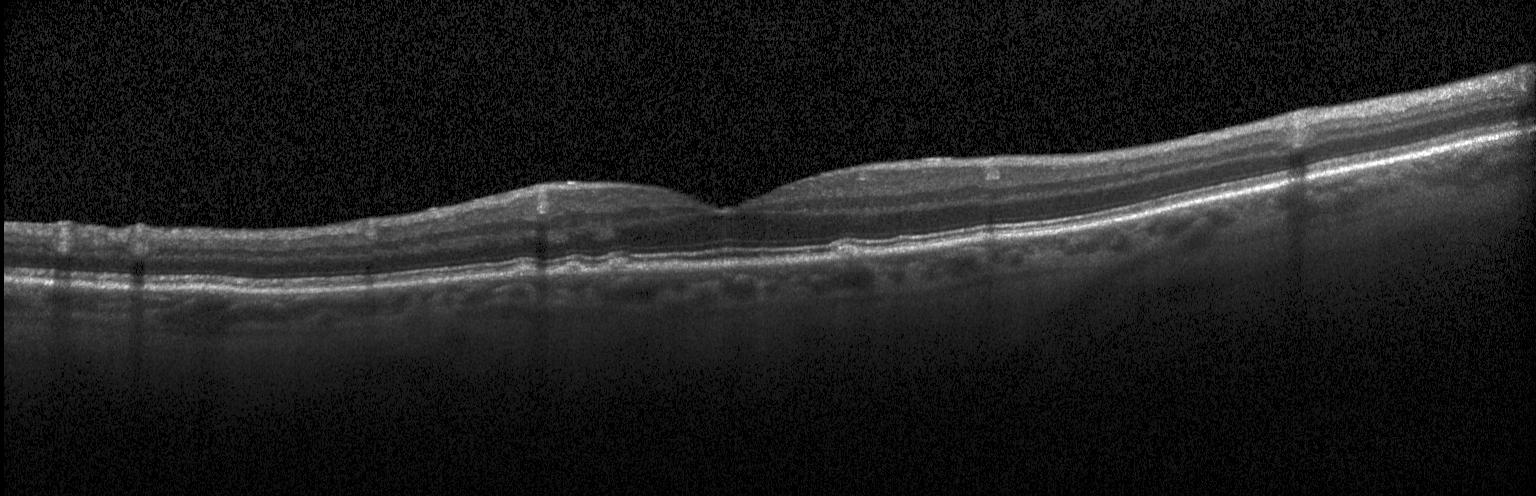
OCT B-scan showing drusen.